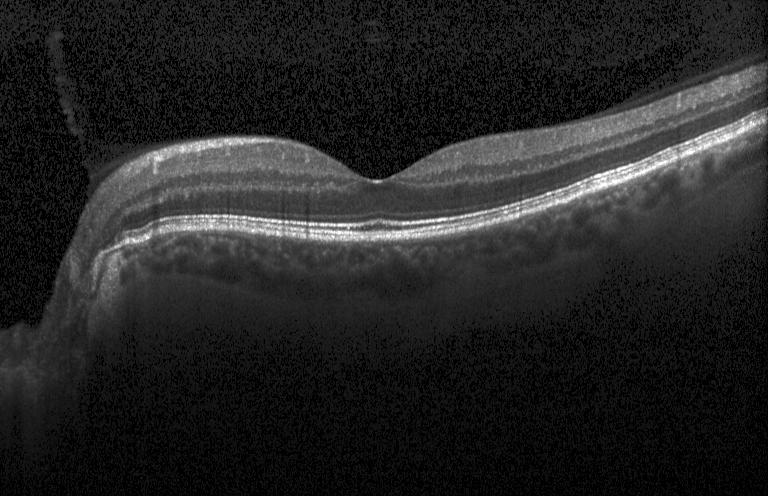
Retinal OCT cross-section showing no evidence of choroidal neovascularization, diabetic macular edema, or drusen.